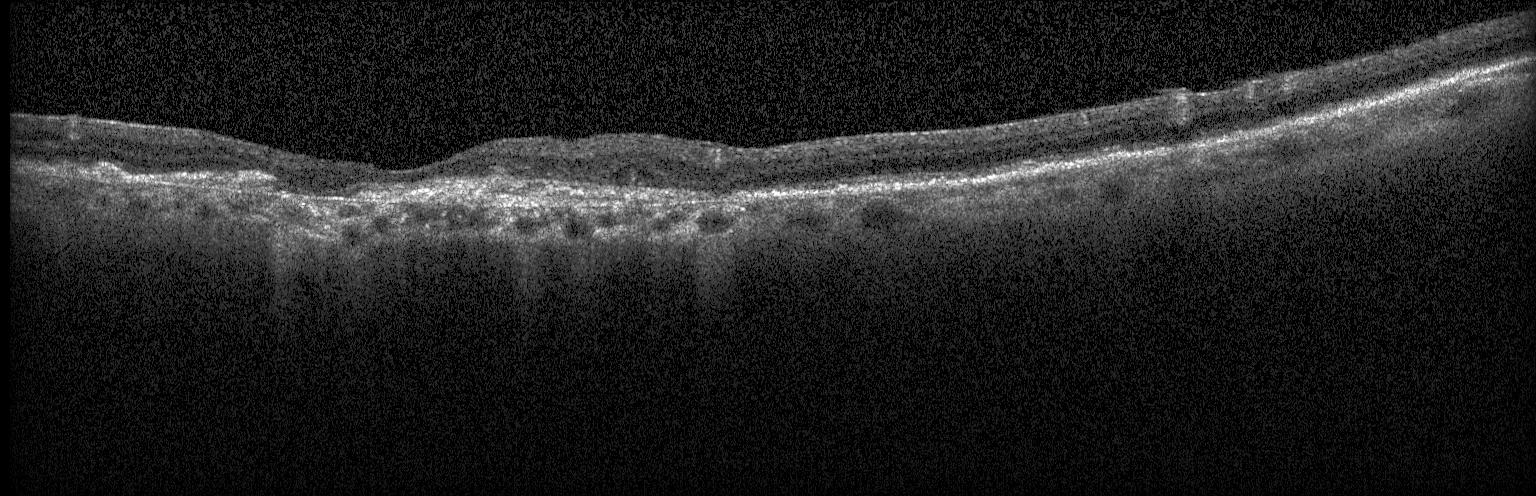
Retinal OCT B-scan. Horizontal scan through the fovea. The scan shows a choroidal neovascular membrane.